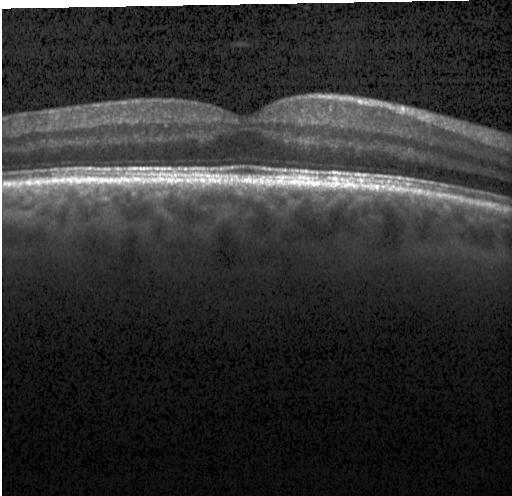 OCT line scan, spectral-domain OCT. Macular OCT: neither CNV, DME, nor drusen.